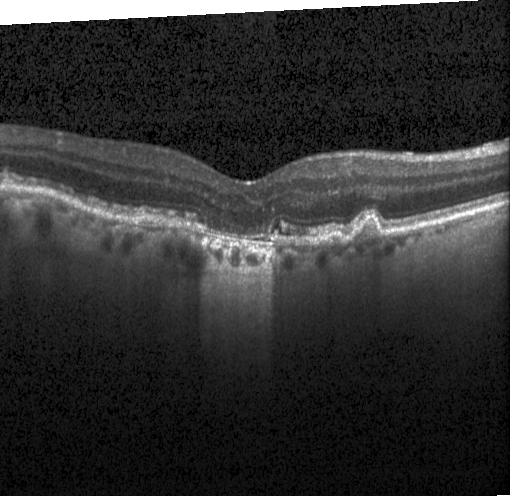
Dx: a choroidal neovascular membrane.